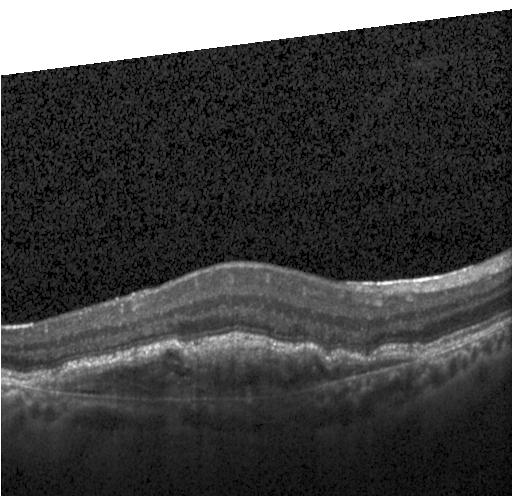
Heidelberg Spectralis OCT system; spectral-domain optical coherence tomography; OCT B-scan; horizontal scan through the fovea. The scan shows a choroidal neovascular membrane.